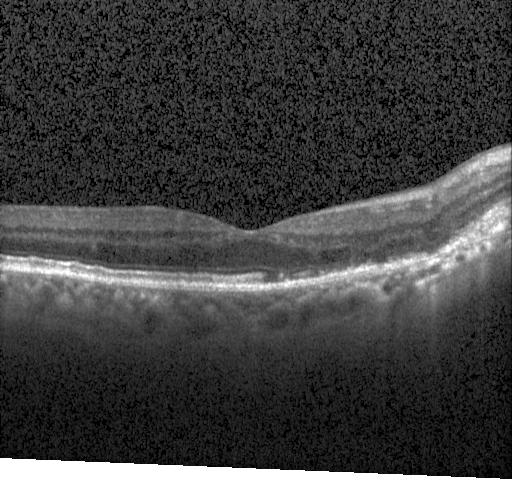

Spectral-domain OCT, retinal OCT cross-section. Diagnosis: CNV.